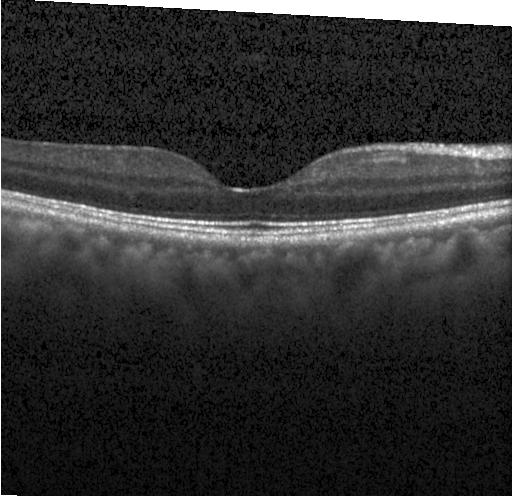

Heidelberg Spectralis OCT system. Spectral-domain optical coherence tomography. Retinal OCT cross-section. Fovea-centered.
Impression: no evidence of choroidal neovascularization, diabetic macular edema, or drusen.